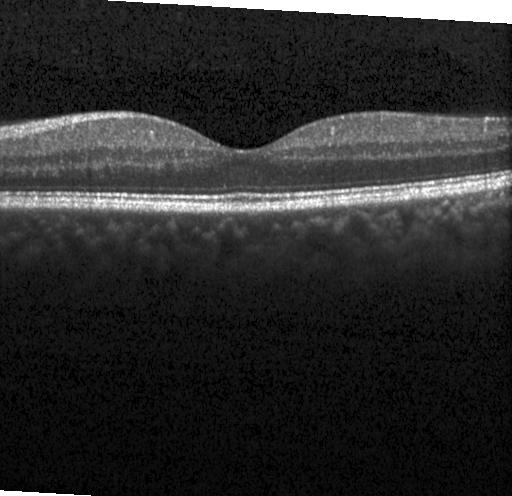 Optical coherence tomography scan — Diagnosis: no CNV, DME, or drusen.